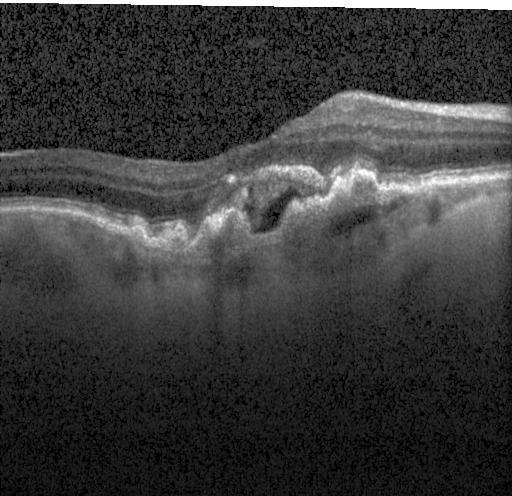
Heidelberg Spectralis OCT system · spectral-domain OCT · optical coherence tomography B-scan · centered on the fovea — Macular OCT: choroidal neovascularization.